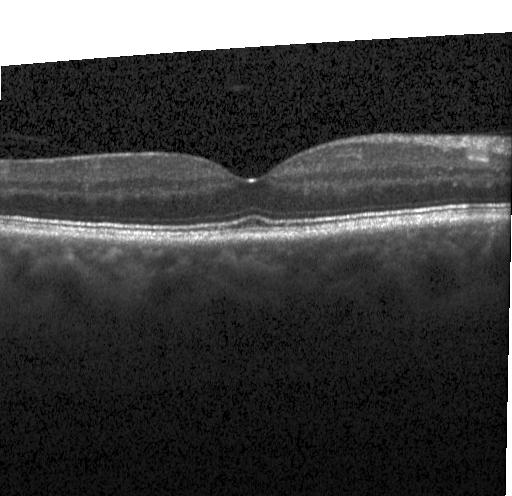 OCT scan showing no evidence of CNV, DME, or drusen.